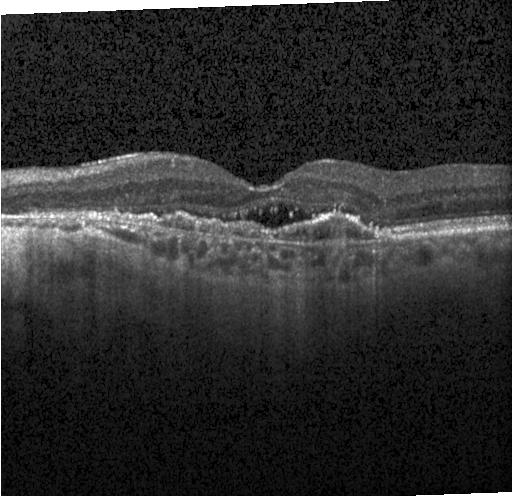

OCT B-scan. Fovea-centered. Finding: CNV.